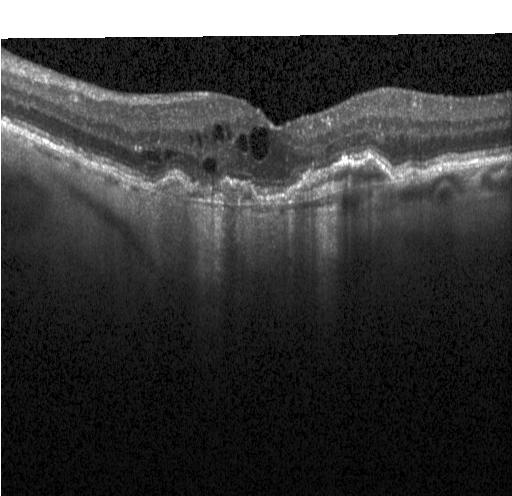 Spectral-domain OCT; optical coherence tomography B-scan; fovea-centered; Heidelberg Spectralis OCT system
Choroidal neovascularization.